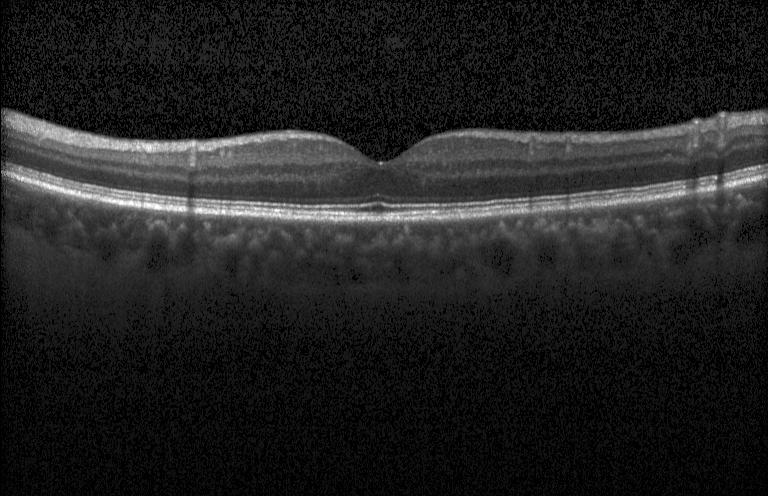

Heidelberg Spectralis OCT system, spectral-domain OCT, optical coherence tomography B-scan, through the macula
Impression: no evidence of CNV, DME, or drusen.